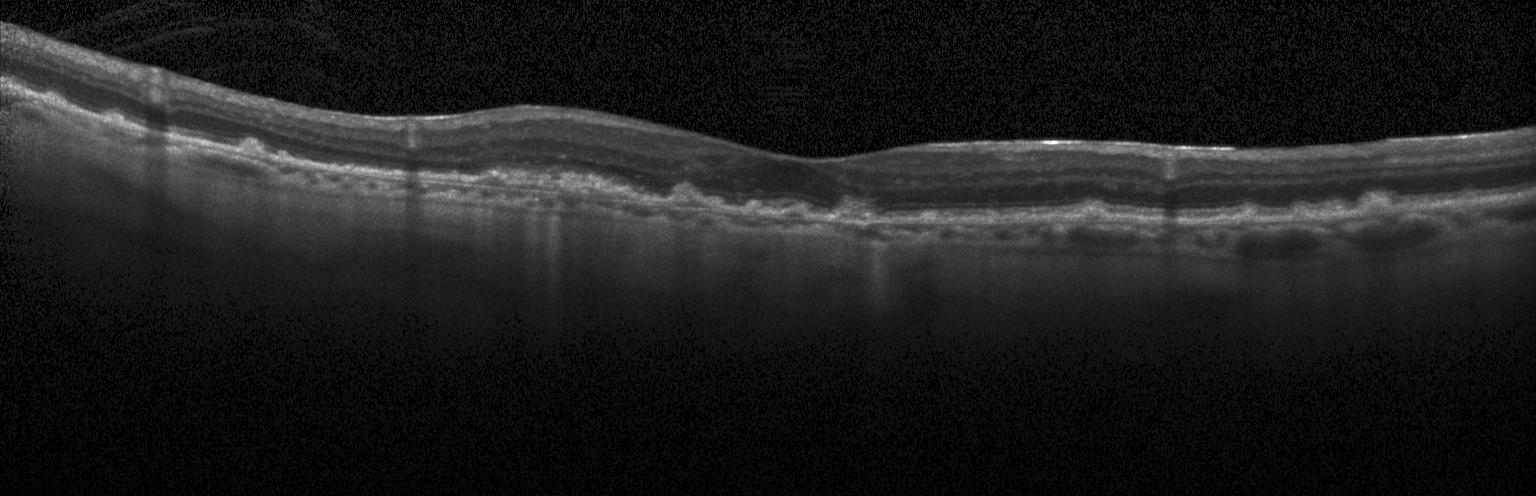
Retinal OCT B-scan. Instrument: Heidelberg Spectralis. Centered on the fovea. Spectral-domain optical coherence tomography
Assessment: a choroidal neovascular membrane.